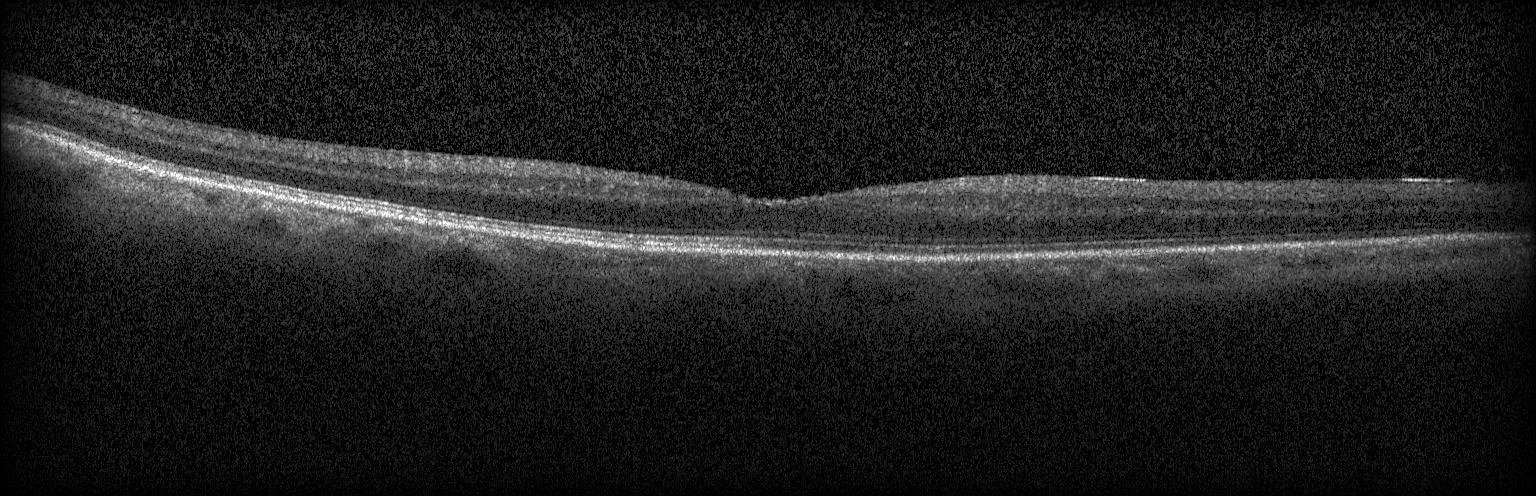 Impression: no CNV, DME, or drusen.